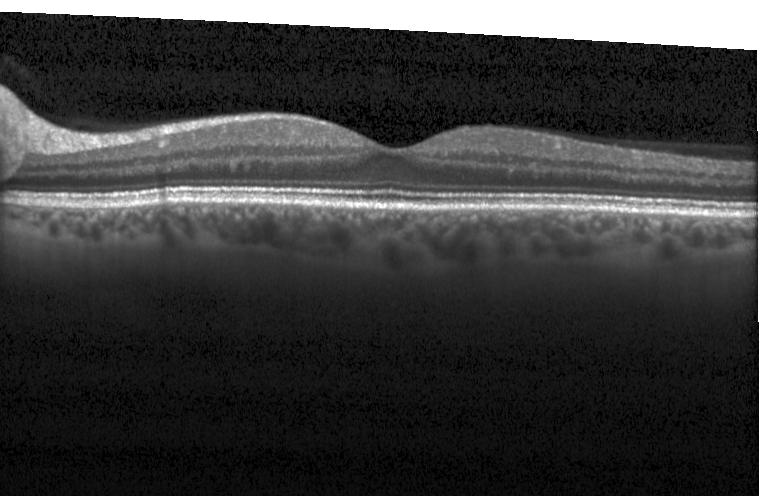
OCT B-scan.
Diagnosis: no evidence of CNV, DME, or drusen.